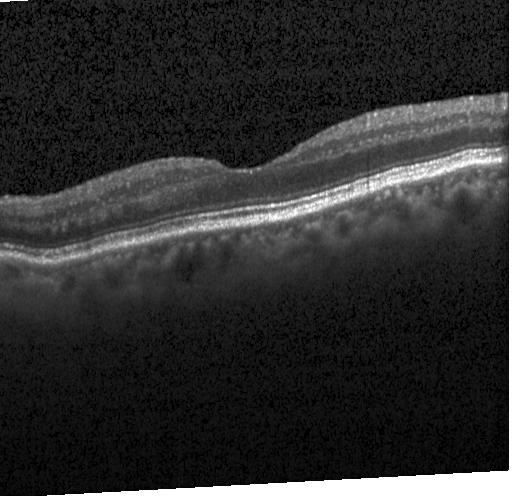
OCT line scan. Through the macula. Spectral-domain OCT — Diagnosis: no CNV, no DME, and no drusen.